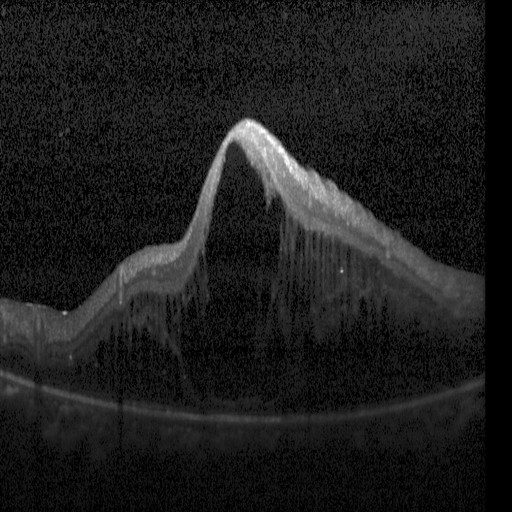 Heidelberg Spectralis OCT system; retinal OCT B-scan; SD-OCT; through the macula.
The scan shows diabetic macular edema.